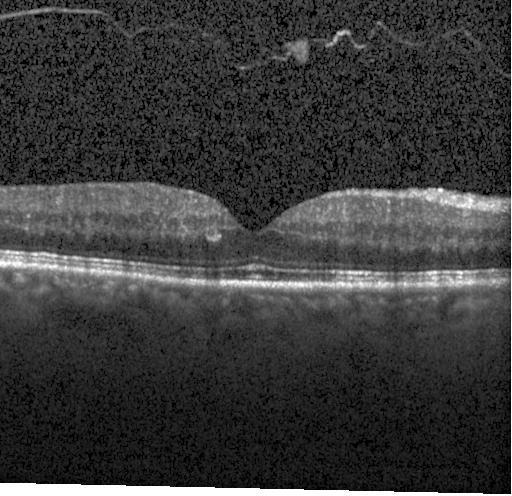
Macular OCT: no evidence of choroidal neovascularization, diabetic macular edema, or drusen.